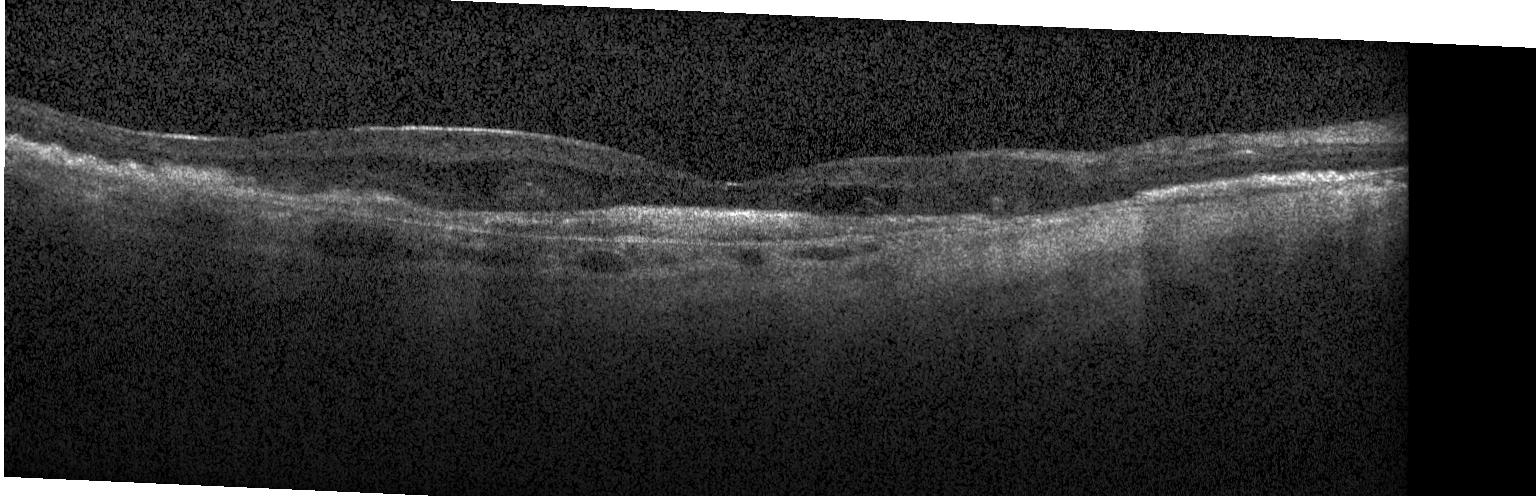 Macular scan · spectral-domain OCT · Heidelberg Spectralis · retinal OCT cross-section — Finding: a choroidal neovascular membrane.